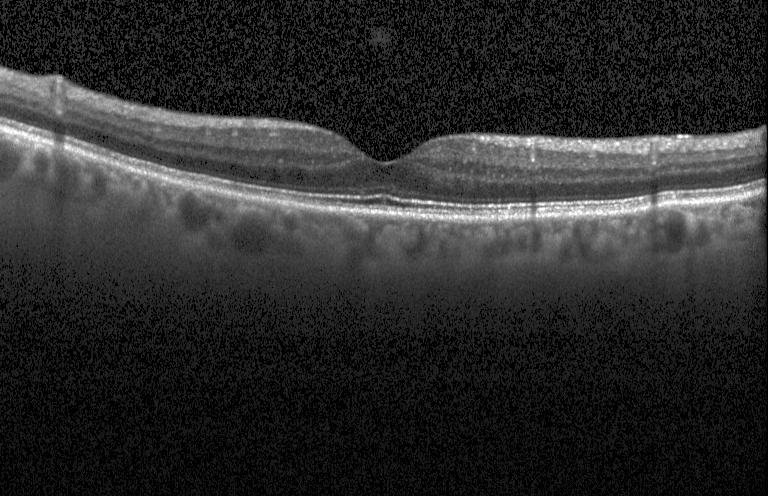
OCT finding: neither CNV, DME, nor drusen.